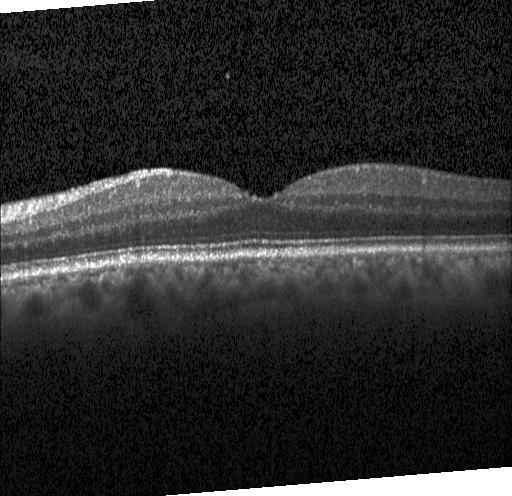

Spectral-domain OCT B-scan: no CNV, no DME, and no drusen.